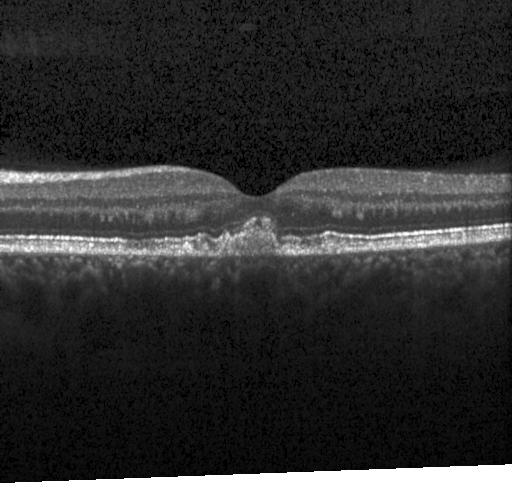 Impression: drusen.